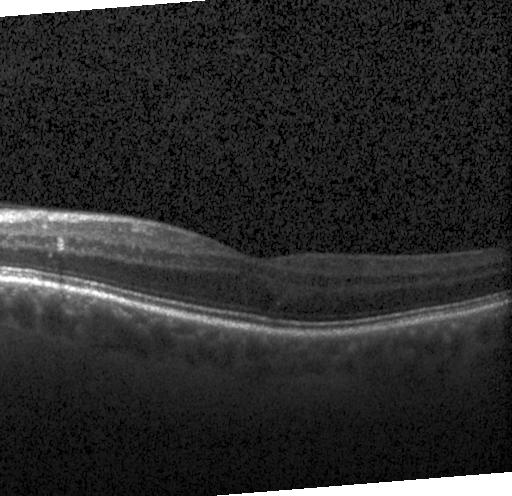

Retinal OCT cross-section. Instrument: Heidelberg Spectralis. Macular scan. Impression: no evidence of choroidal neovascularization, diabetic macular edema, or drusen.